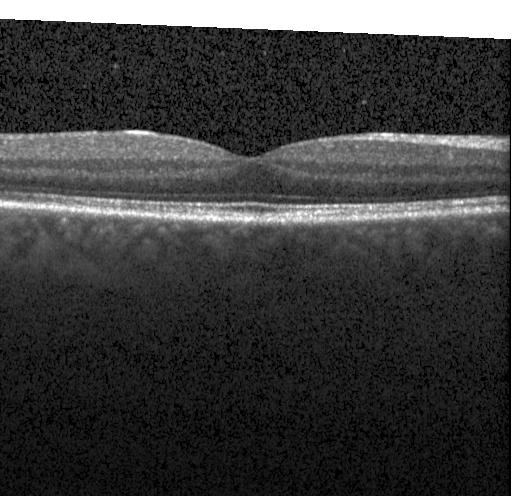

Optical coherence tomography scan, through the macula
Neither choroidal neovascularization, diabetic macular edema, nor drusen.